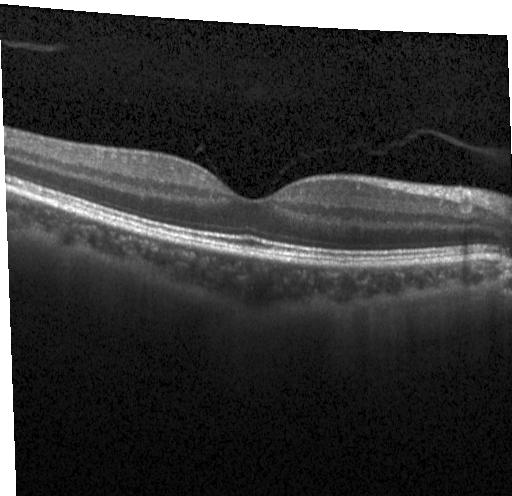
OCT finding: neither choroidal neovascularization, diabetic macular edema, nor drusen.